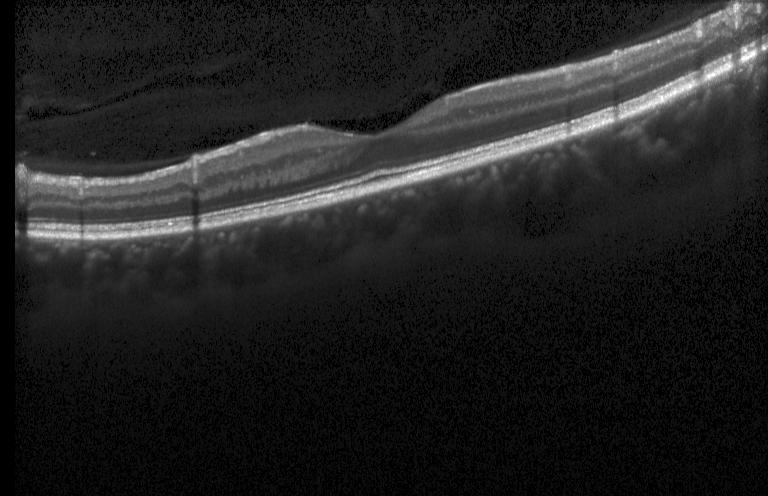

OCT line scan · SD-OCT · Heidelberg Spectralis OCT system.
Finding: no evidence of choroidal neovascularization, diabetic macular edema, or drusen.